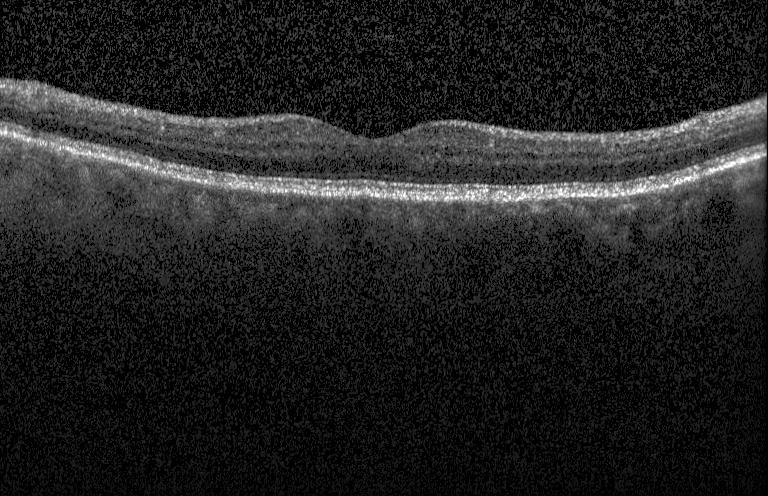

Dx: no choroidal neovascularization, diabetic macular edema, or drusen.